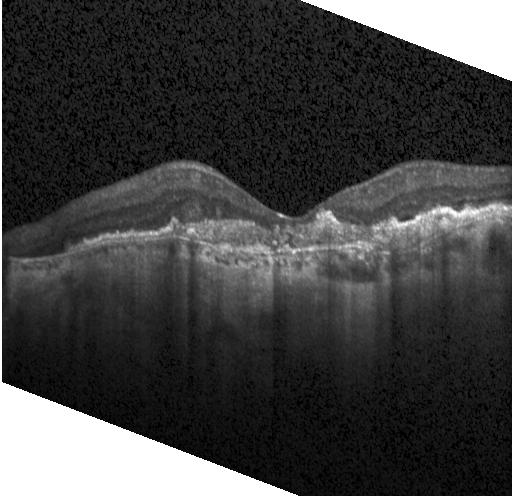
Macular OCT demonstrating CNV.